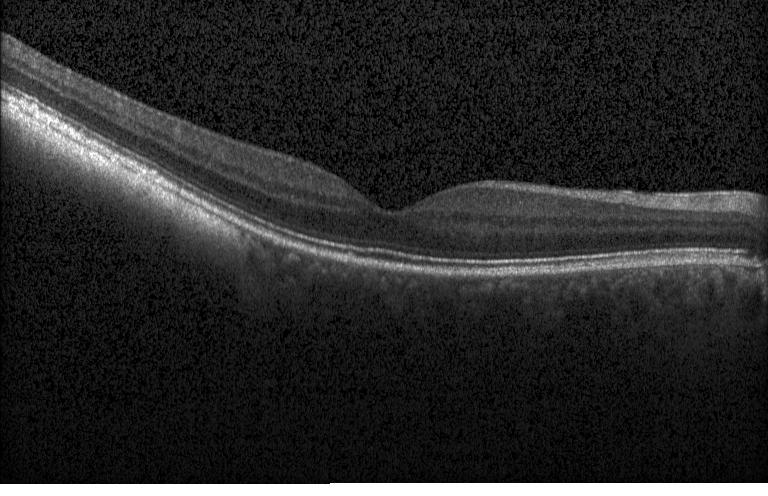 Impression: drusen.